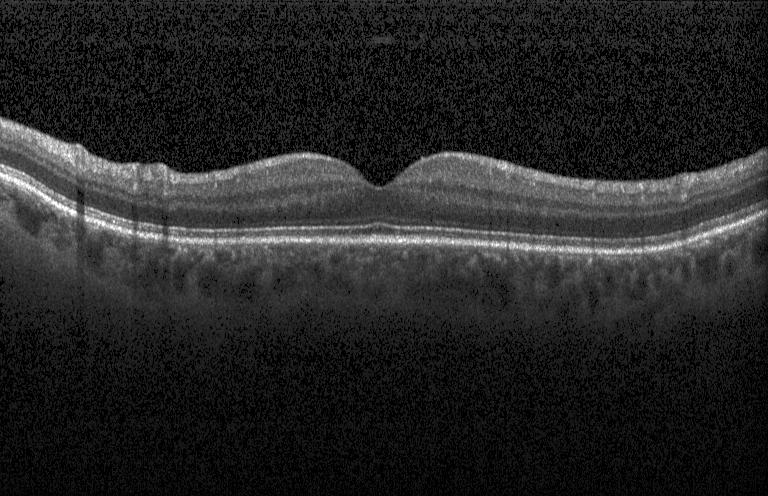
OCT B-scan — The scan shows no evidence of choroidal neovascularization, diabetic macular edema, or drusen.